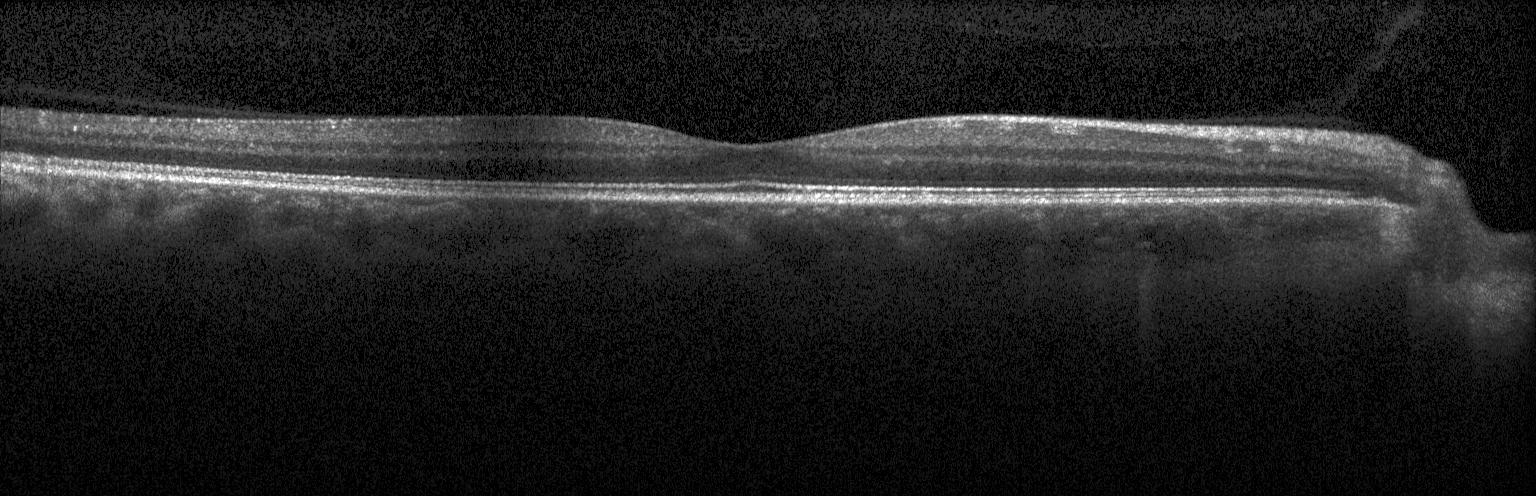
Acquired on a Heidelberg Spectralis, retinal OCT cross-section — The scan shows no choroidal neovascularization, diabetic macular edema, or drusen.